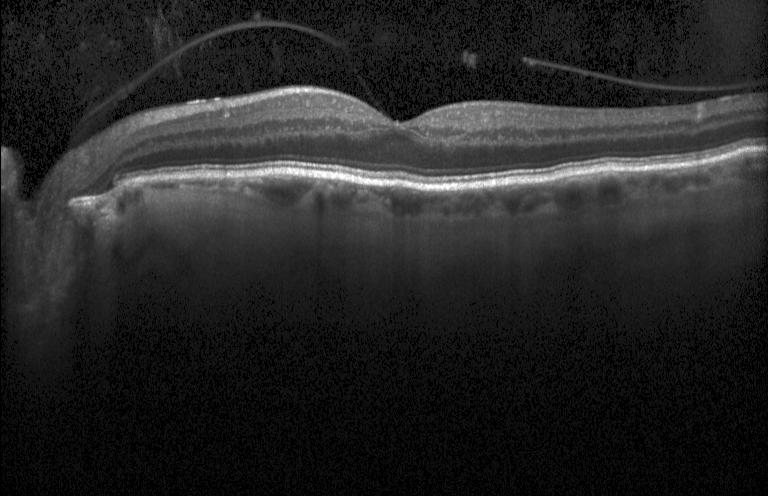
Optical coherence tomography B-scan; instrument: Heidelberg Spectralis.
Finding: neither choroidal neovascularization, diabetic macular edema, nor drusen.